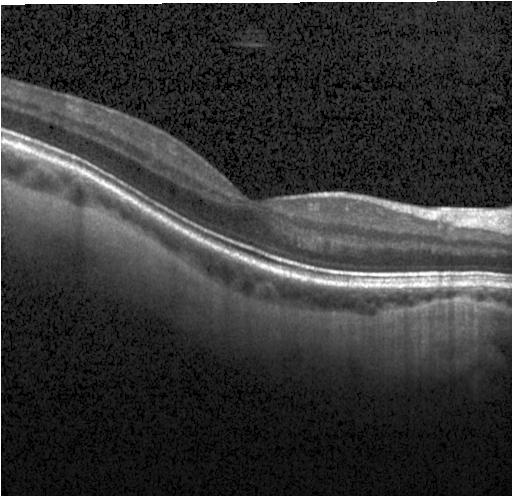

Optical coherence tomography B-scan · instrument: Heidelberg Spectralis · through the macula · SD-OCT
The scan shows no evidence of CNV, DME, or drusen.